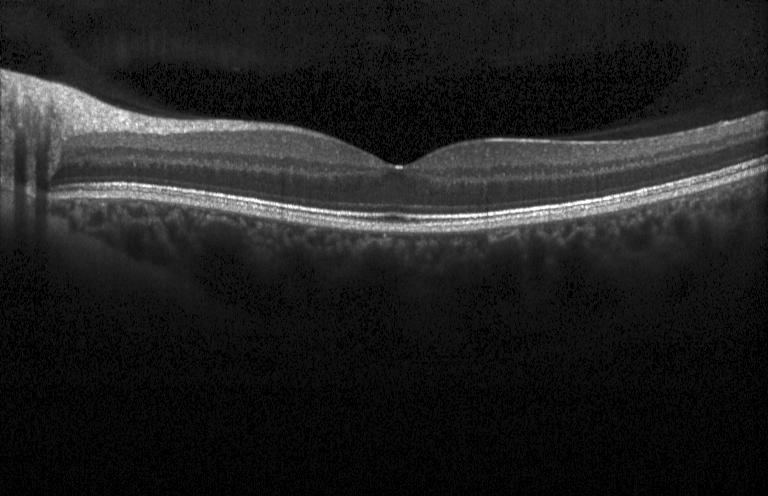 Dx: no choroidal neovascularization, no diabetic macular edema, and no drusen.